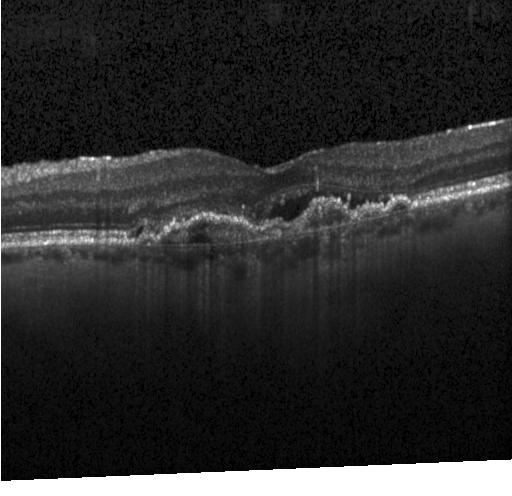 Through the macula; spectral-domain OCT; OCT line scan — Assessment: CNV.